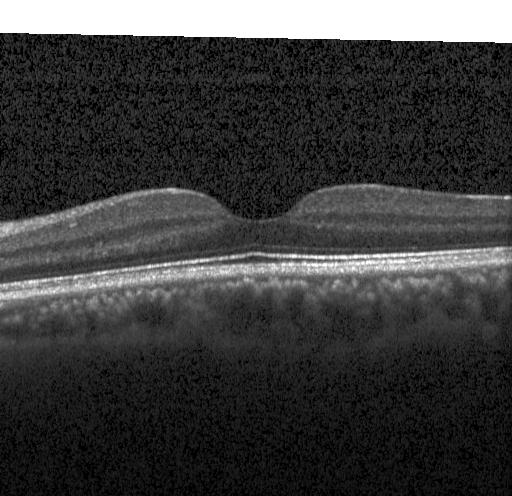

Spectral-domain OCT B-scan: no evidence of choroidal neovascularization, diabetic macular edema, or drusen.